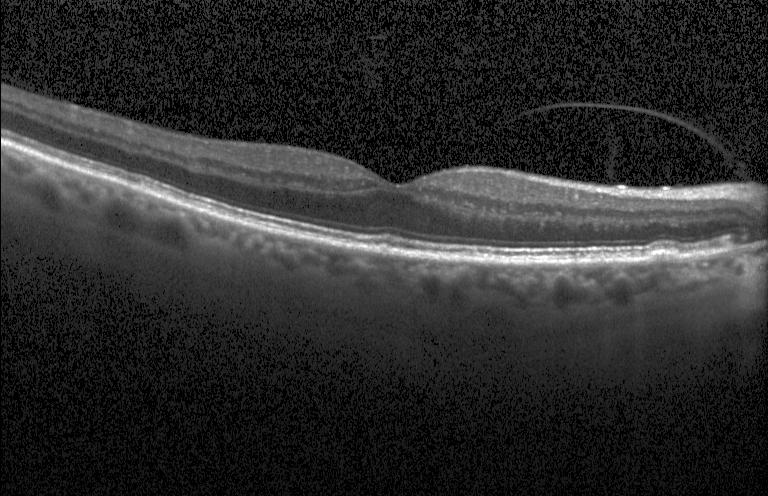 Optical coherence tomography scan; spectral-domain OCT; Heidelberg Spectralis OCT system; through the macula — Diagnosis: neither choroidal neovascularization, diabetic macular edema, nor drusen.